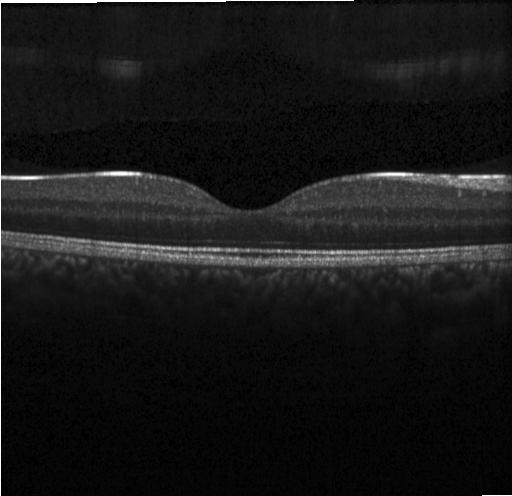 OCT scan showing no choroidal neovascularization, no diabetic macular edema, and no drusen.